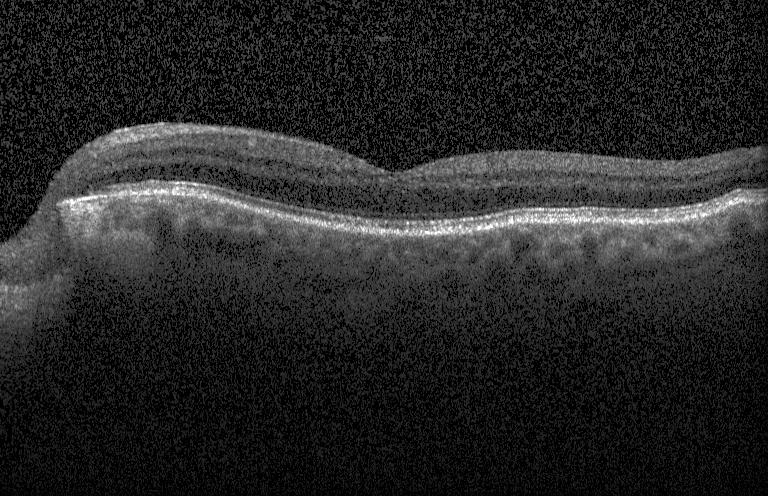

Finding: neither choroidal neovascularization, diabetic macular edema, nor drusen.